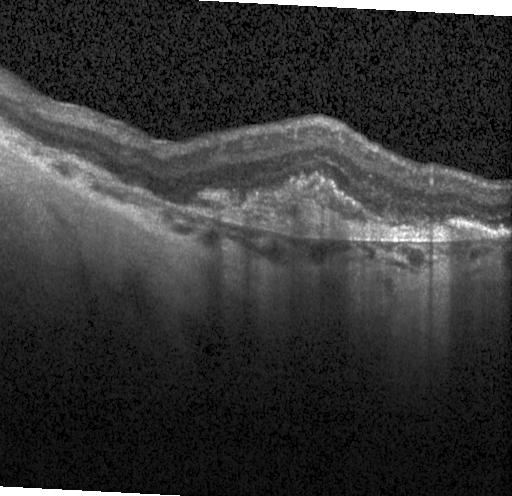

Instrument: Heidelberg Spectralis; retinal OCT cross-section — Dx: a choroidal neovascular membrane.